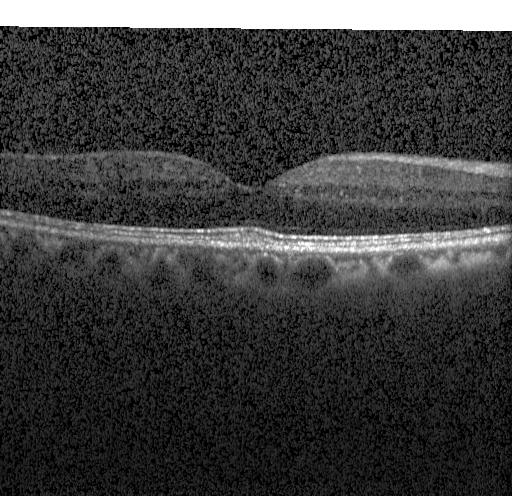

Spectral-domain OCT B-scan: no choroidal neovascularization, diabetic macular edema, or drusen.